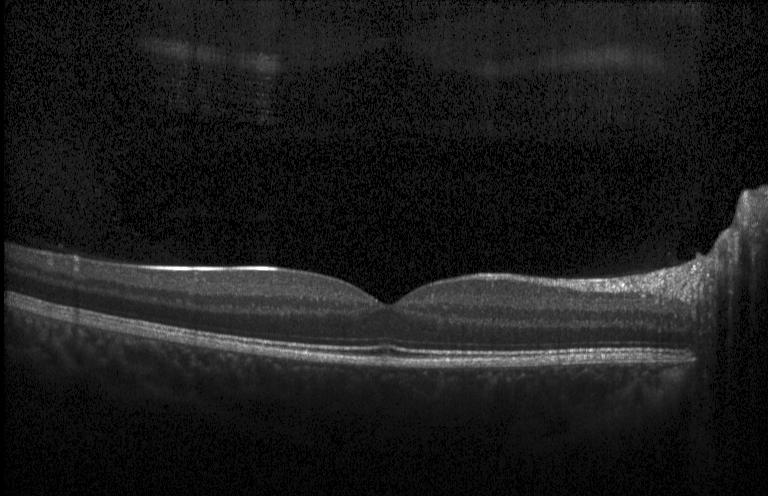
The scan shows no CNV, no DME, and no drusen.